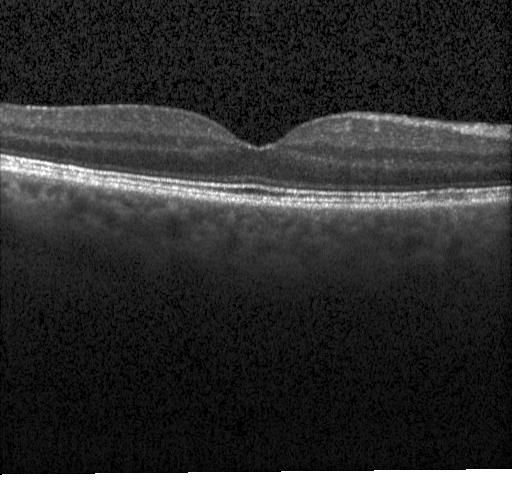 Macular OCT demonstrating no CNV, no DME, and no drusen.